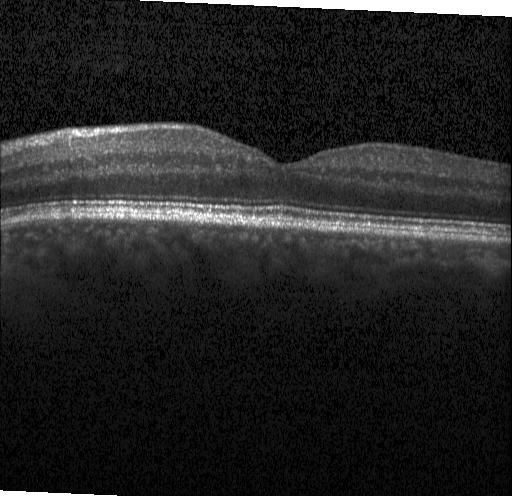 Finding: no choroidal neovascularization, no diabetic macular edema, and no drusen.